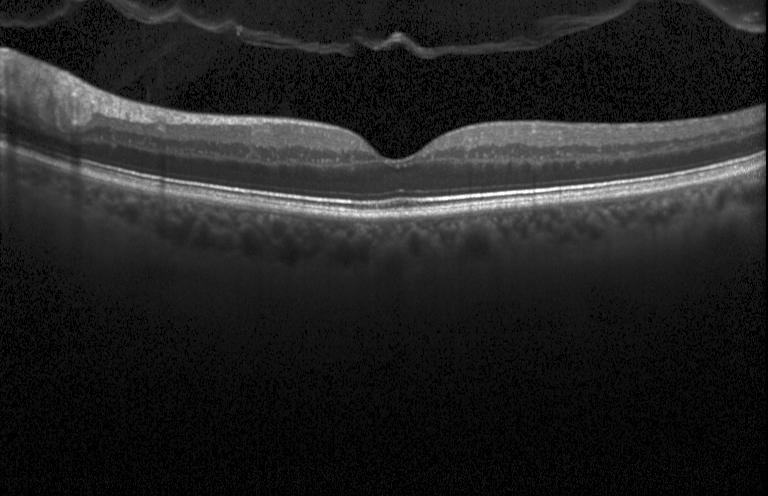 OCT line scan
Diagnosis: no choroidal neovascularization, diabetic macular edema, or drusen.